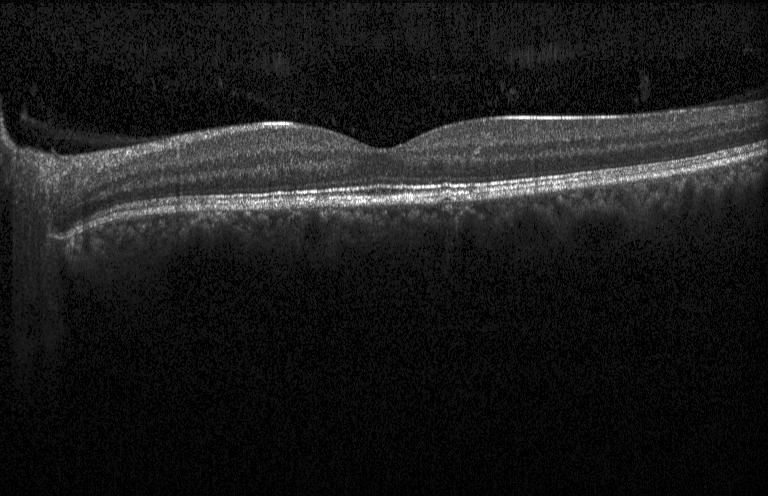
Instrument: Heidelberg Spectralis · macular scan · retinal OCT B-scan · spectral-domain OCT. Finding: no evidence of CNV, DME, or drusen.